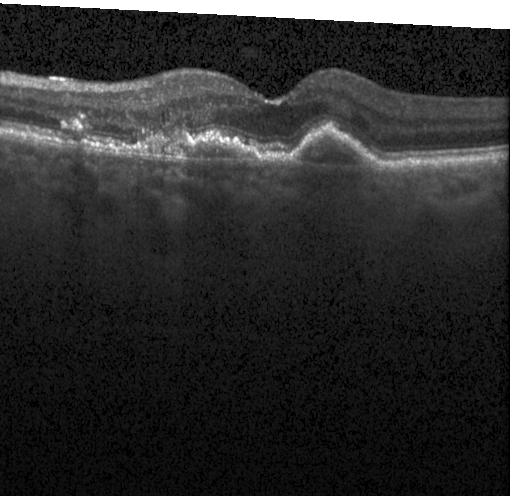 OCT B-scan; acquired on a Heidelberg Spectralis
Diagnosis: choroidal neovascularization (CNV).